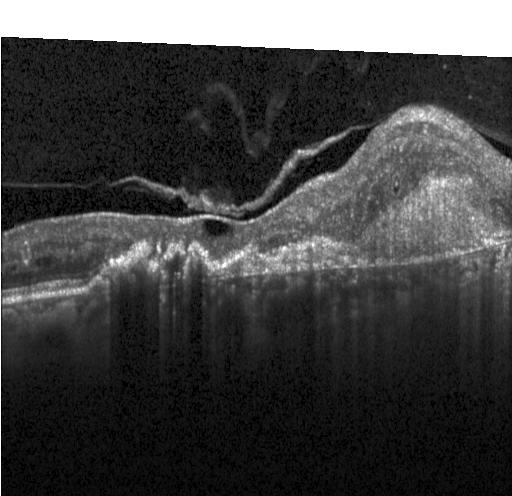
Diagnosis: a choroidal neovascular membrane.